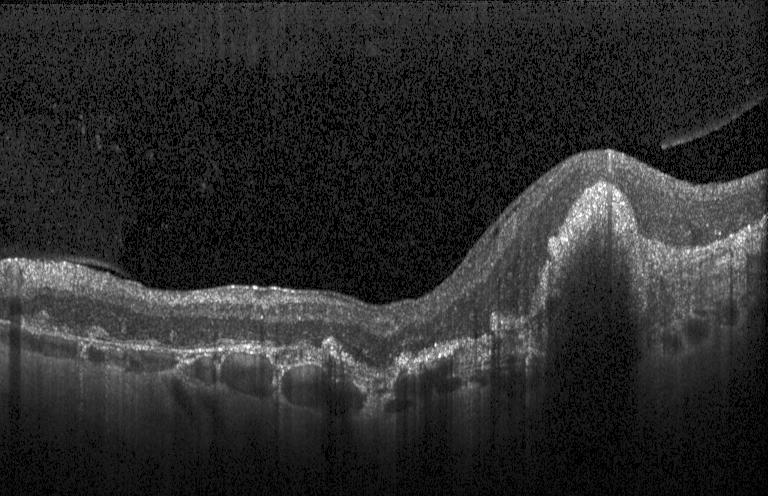
OCT line scan.
Impression: choroidal neovascularization (CNV).